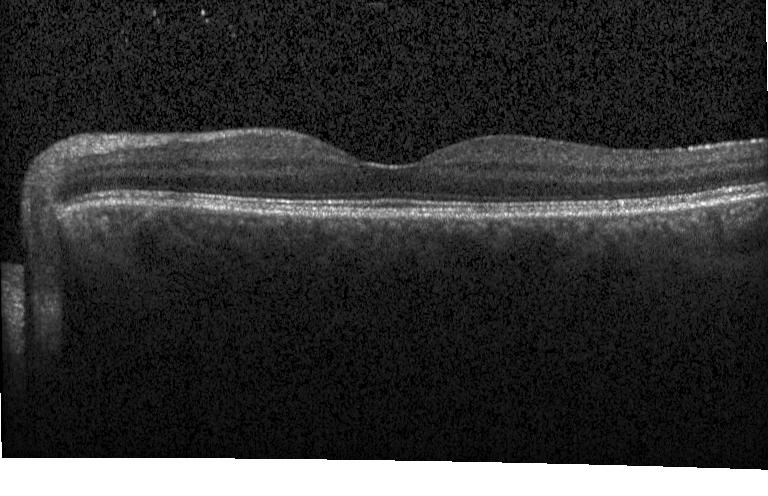 Macular scan; OCT line scan
Impression: no evidence of choroidal neovascularization, diabetic macular edema, or drusen.